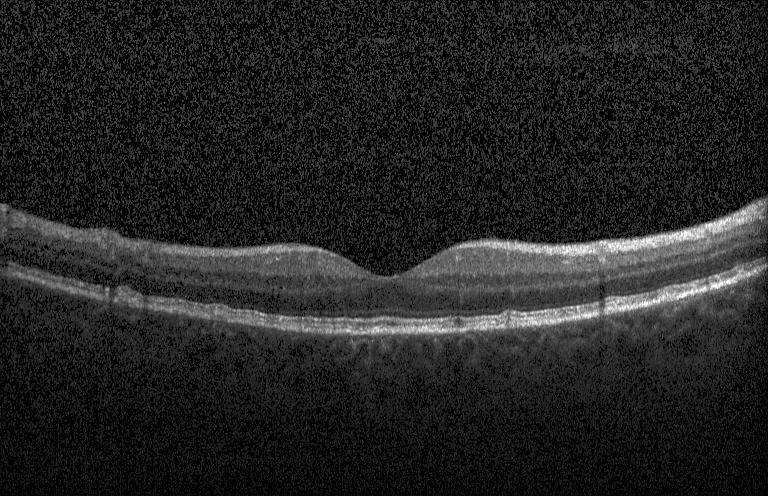

OCT B-scan
Impression: sub-RPE drusenoid deposits.